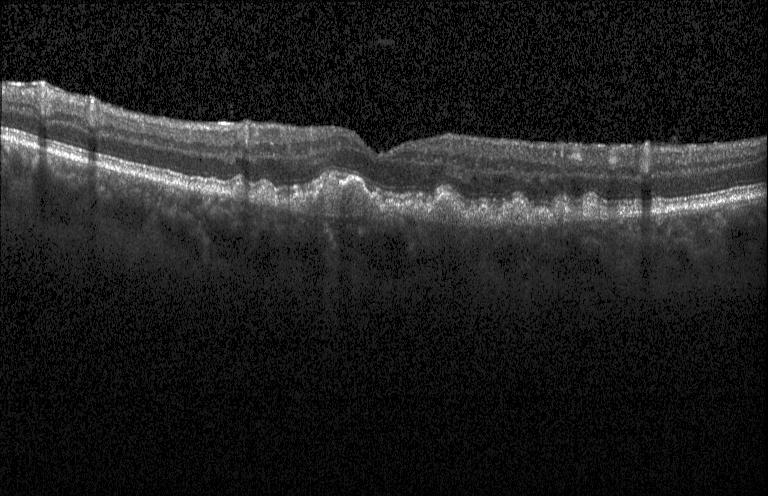
Optical coherence tomography B-scan — Diagnosis: choroidal neovascularization (CNV).